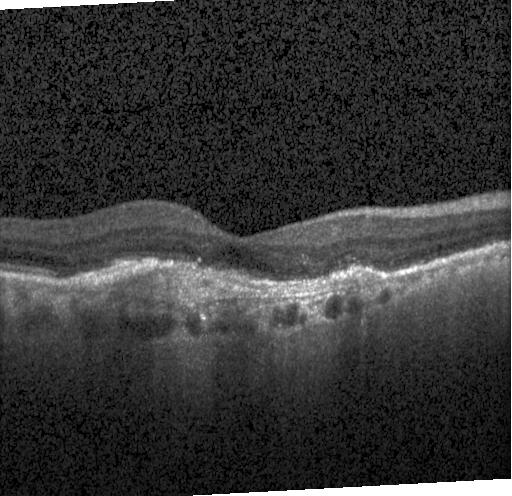 OCT line scan. Horizontal scan through the fovea. Spectral-domain OCT. Acquired on a Heidelberg Spectralis — Impression: choroidal neovascularization (CNV).